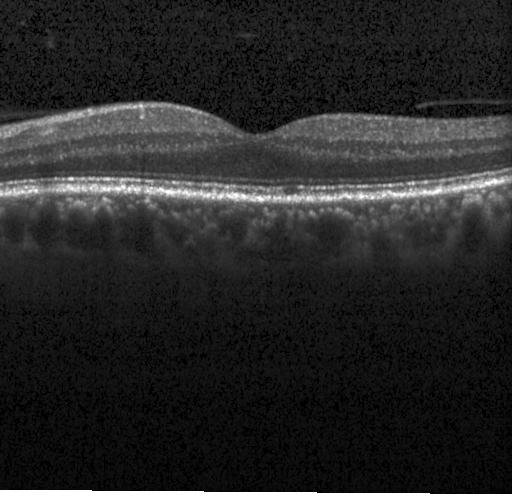
Diagnosis: no evidence of choroidal neovascularization, diabetic macular edema, or drusen.